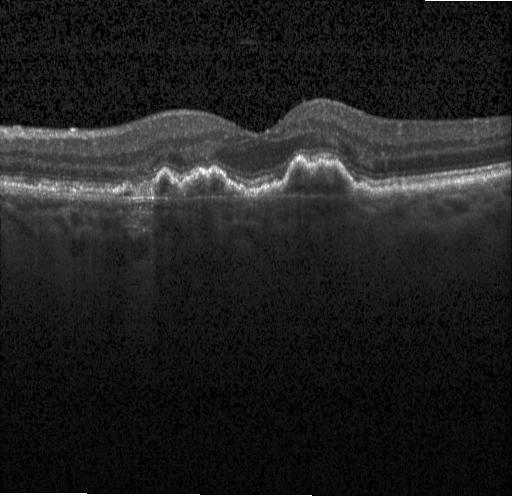
Spectral-domain OCT. Acquired on a Heidelberg Spectralis. Macular scan. OCT line scan
Impression: a choroidal neovascular membrane.